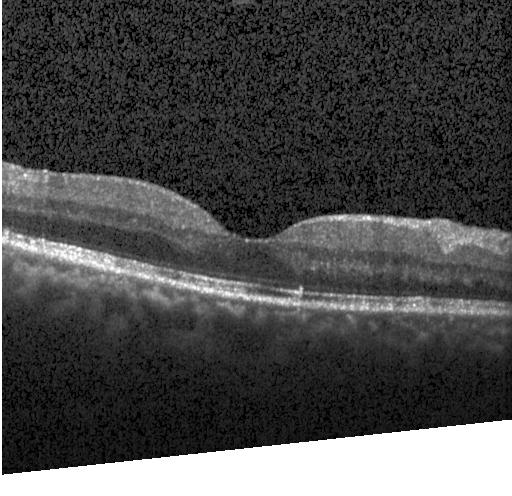

Optical coherence tomography scan, spectral-domain optical coherence tomography, instrument: Heidelberg Spectralis.
Impression: no evidence of choroidal neovascularization, diabetic macular edema, or drusen.